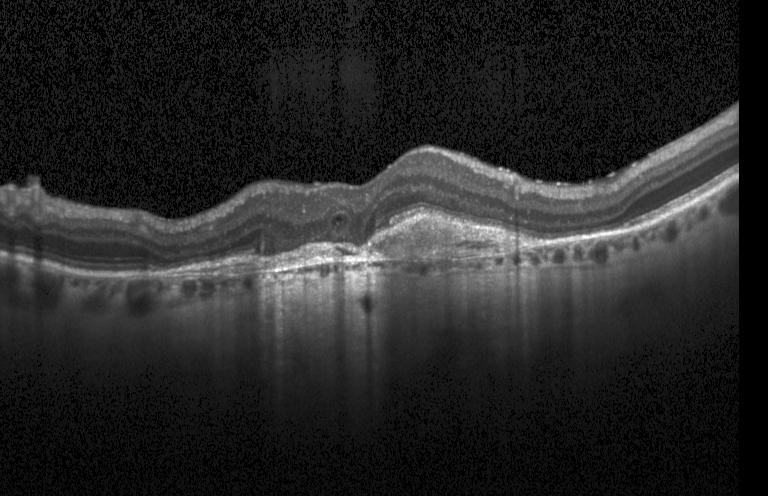

Optical coherence tomography B-scan, Heidelberg Spectralis OCT system, spectral-domain OCT. Dx: choroidal neovascularization (CNV).